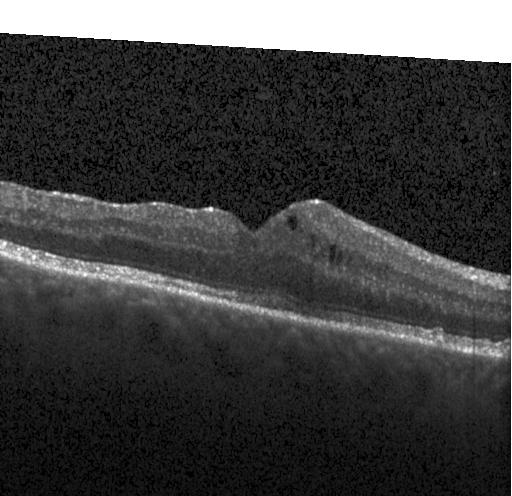
Finding: diabetic macular edema (DME).